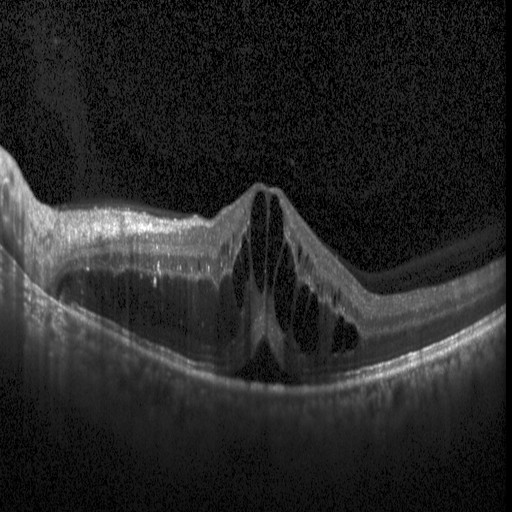 Spectral-domain OCT B-scan: diabetic macular edema (DME).